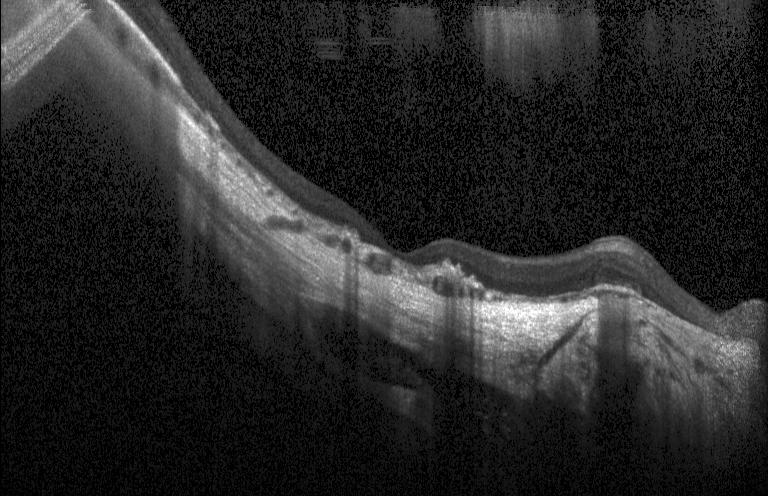 Heidelberg Spectralis. Retinal OCT B-scan
A choroidal neovascular membrane.